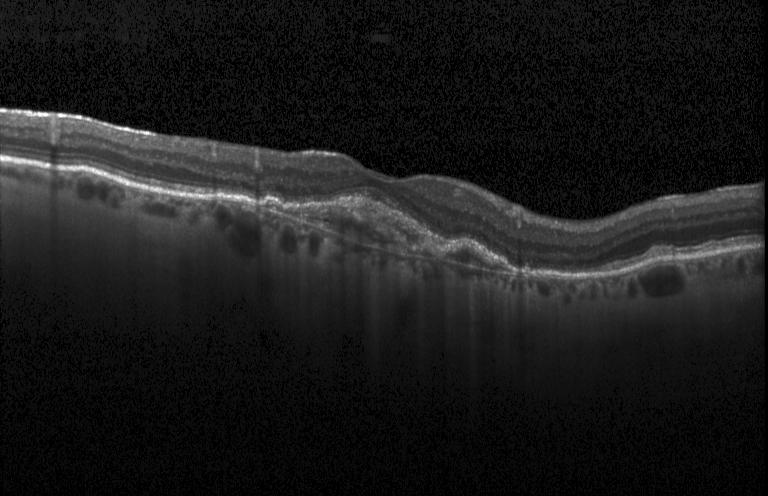
Macular OCT demonstrating choroidal neovascularization.